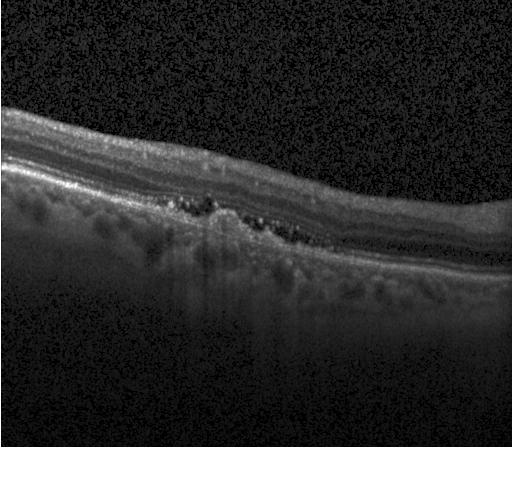 Fovea-centered; optical coherence tomography B-scan; Heidelberg Spectralis — Finding: CNV.